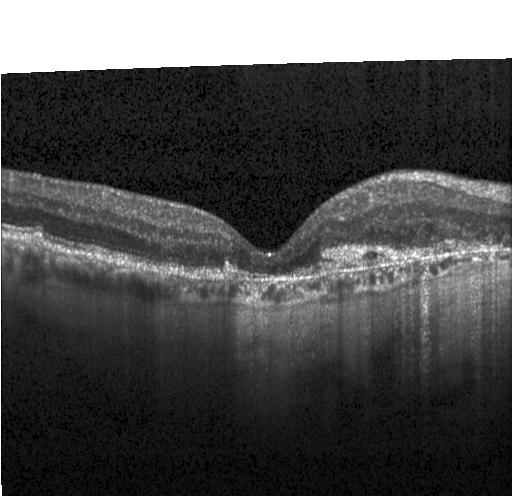 Optical coherence tomography scan · macular scan · acquired on a Heidelberg Spectralis. The scan shows a choroidal neovascular membrane.